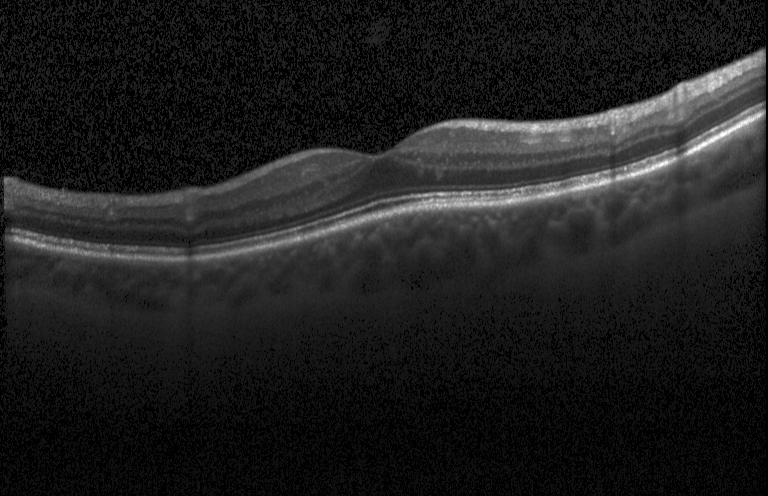
Macular OCT demonstrating no CNV, no DME, and no drusen.